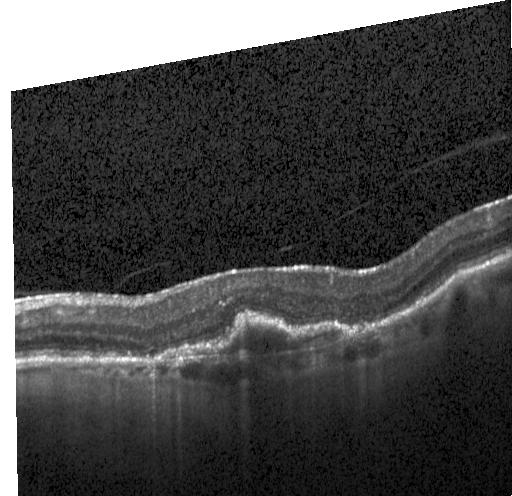

Horizontal scan through the fovea. Retinal OCT cross-section. Spectral-domain OCT. The scan shows CNV.